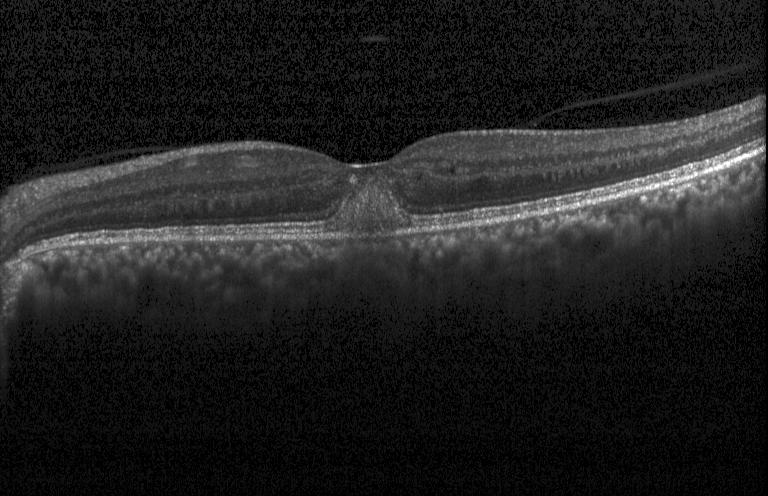 Diagnosis: CNV.